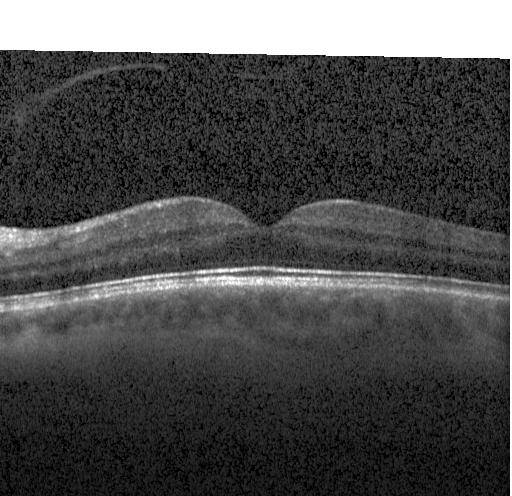
No choroidal neovascularization, no diabetic macular edema, and no drusen.